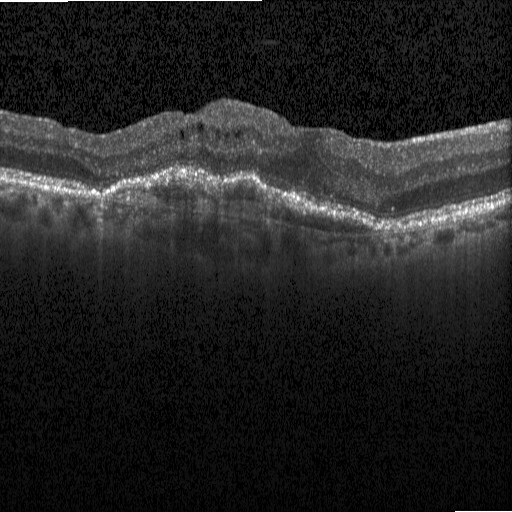
This B-scan demonstrates DME.